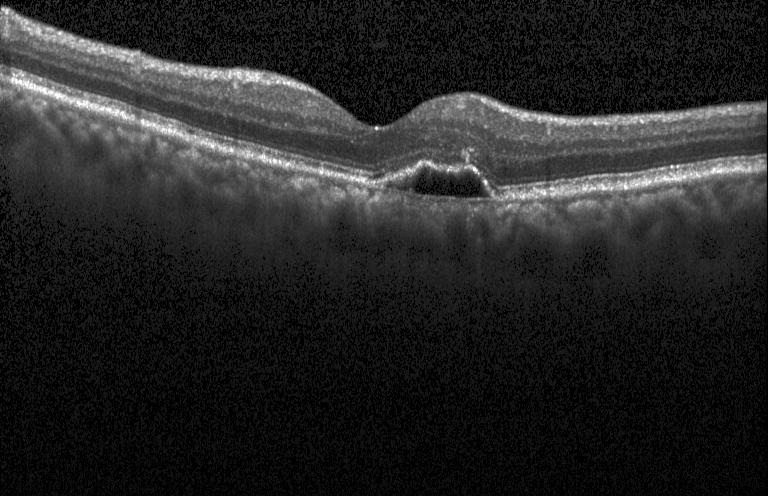 Spectral-domain OCT, macular scan, optical coherence tomography B-scan. Assessment: choroidal neovascularization.